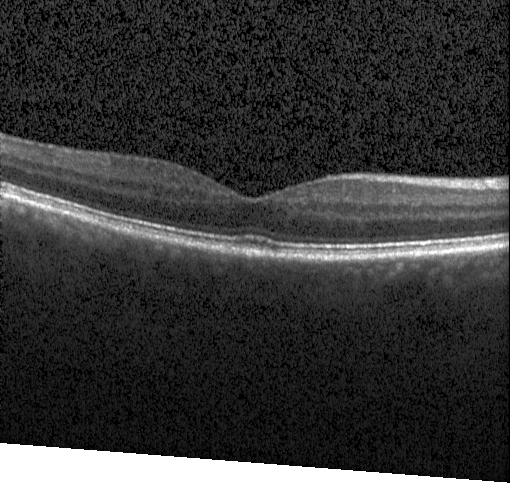

OCT line scan. No CNV, DME, or drusen.